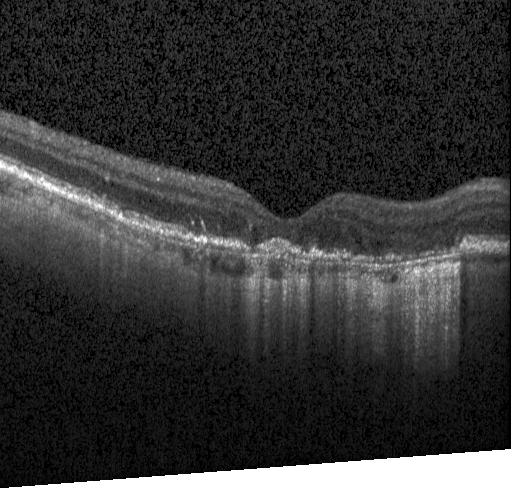
Heidelberg Spectralis. Optical coherence tomography B-scan. Spectral-domain OCT. Through the macula
Assessment: choroidal neovascularization.